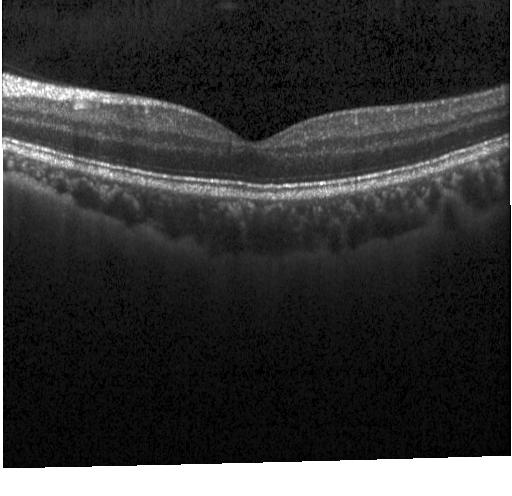

OCT line scan. Diagnosis: neither CNV, DME, nor drusen.